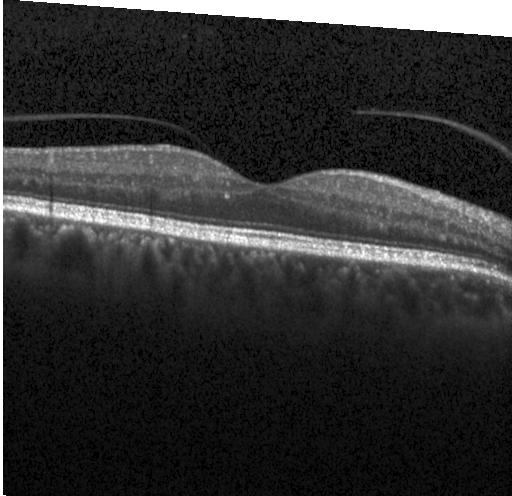 The scan shows no evidence of choroidal neovascularization, diabetic macular edema, or drusen.